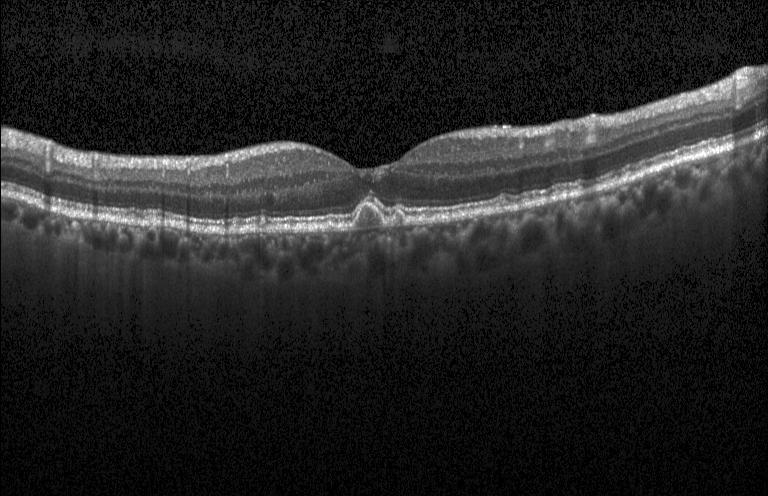
OCT B-scan, Heidelberg Spectralis OCT system, spectral-domain OCT
Assessment: multiple drusen.